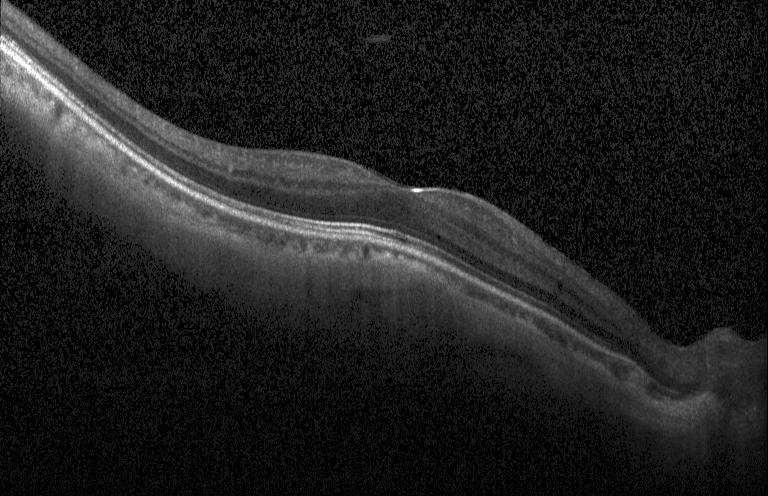

No evidence of CNV, DME, or drusen.